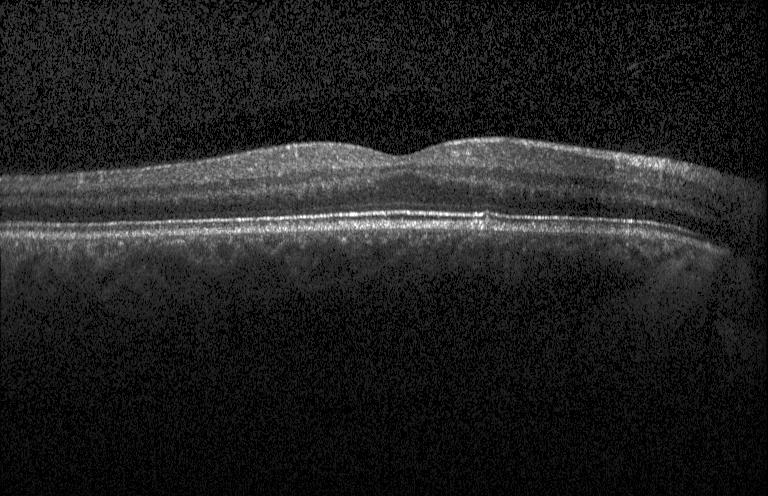 Retinal OCT B-scan. This B-scan demonstrates neither CNV, DME, nor drusen.